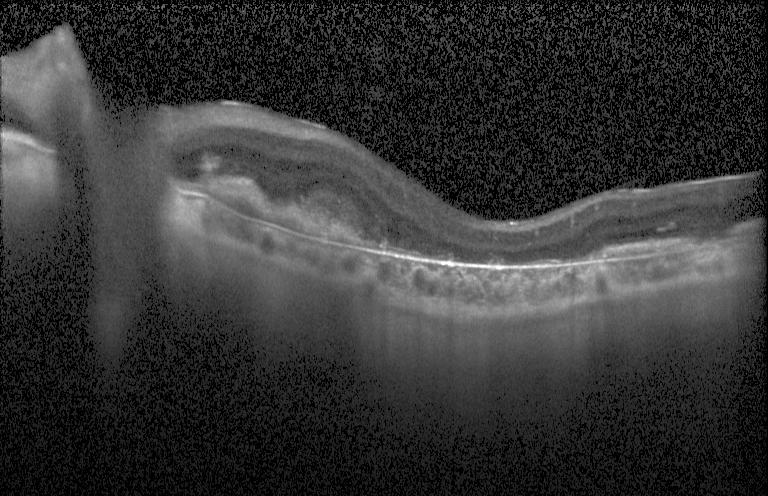 Optical coherence tomography B-scan
Diagnosis: a choroidal neovascular membrane.